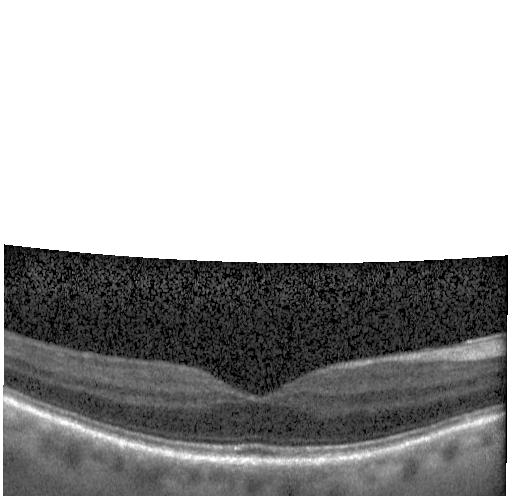 Dx: no evidence of CNV, DME, or drusen.